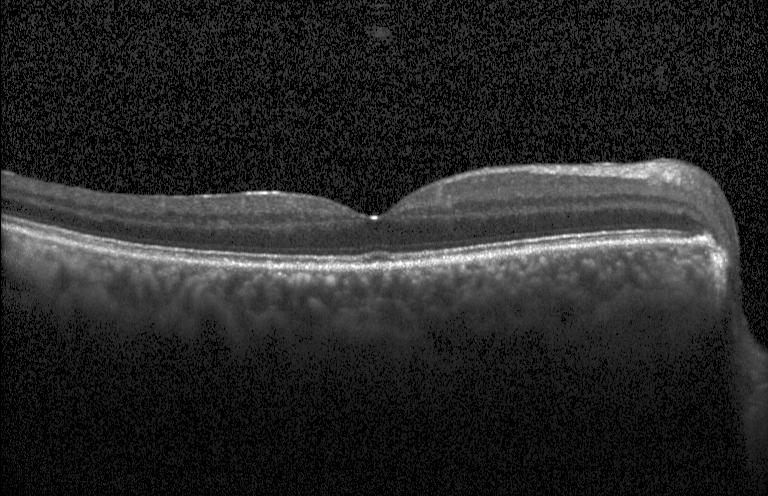
SD-OCT · optical coherence tomography scan
Diagnosis: no evidence of CNV, DME, or drusen.